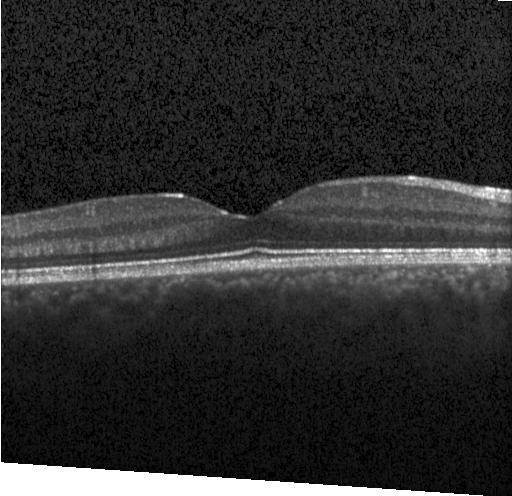

Heidelberg Spectralis OCT system. Optical coherence tomography B-scan. Dx: no CNV, DME, or drusen.